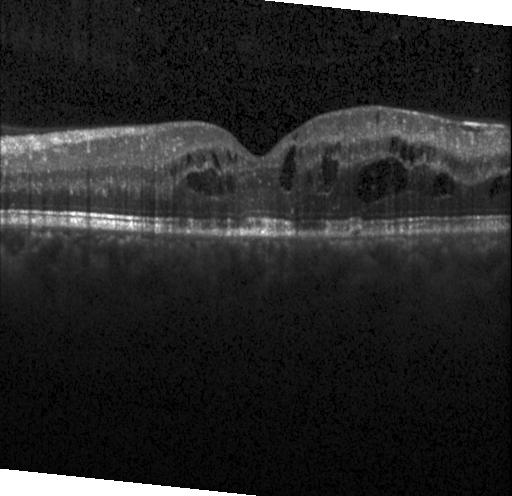
Heidelberg Spectralis, optical coherence tomography B-scan, spectral-domain OCT. Impression: diabetic macular edema.